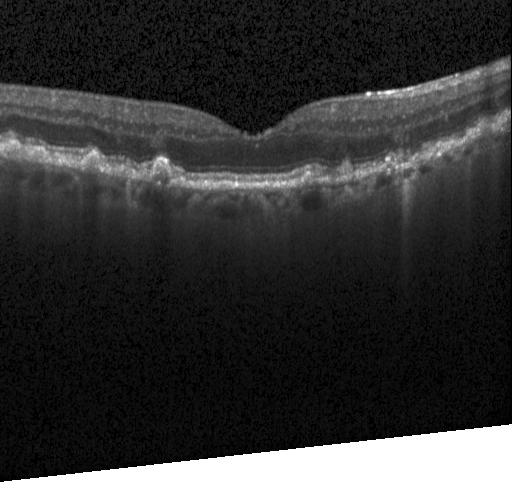
Macular OCT demonstrating sub-RPE drusenoid deposits.